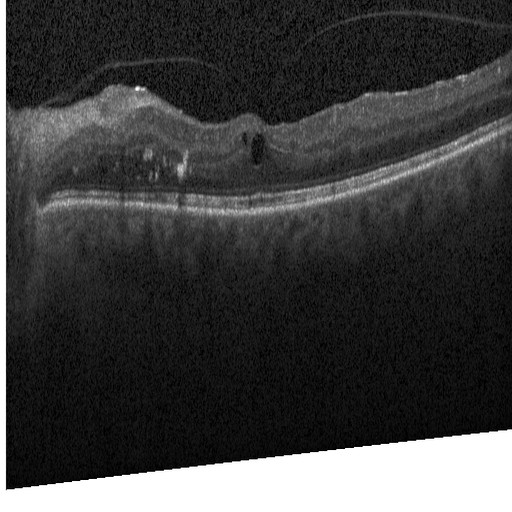
Macular OCT: diabetic macular edema.